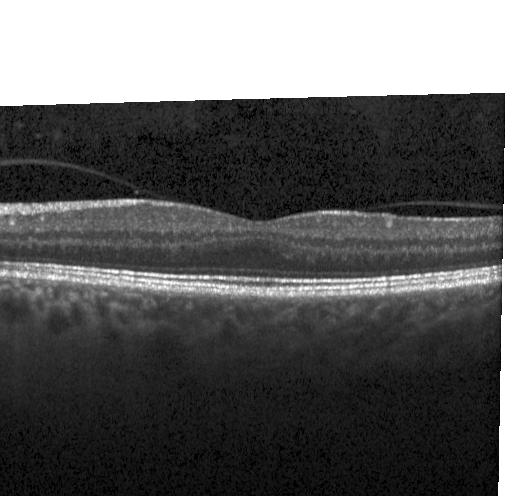
Instrument: Heidelberg Spectralis; OCT line scan.
The scan shows no choroidal neovascularization, no diabetic macular edema, and no drusen.